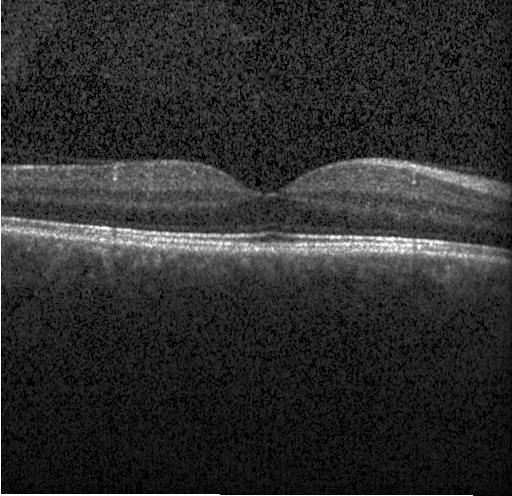
Impression: neither choroidal neovascularization, diabetic macular edema, nor drusen.